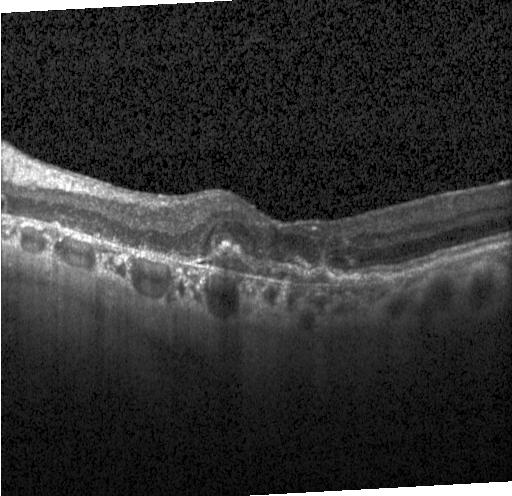

Optical coherence tomography B-scan. Instrument: Heidelberg Spectralis. Through the macula.
Dx: CNV.